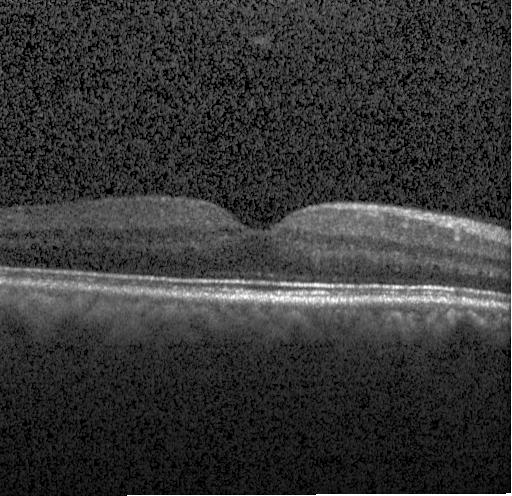

The scan shows no CNV, DME, or drusen.